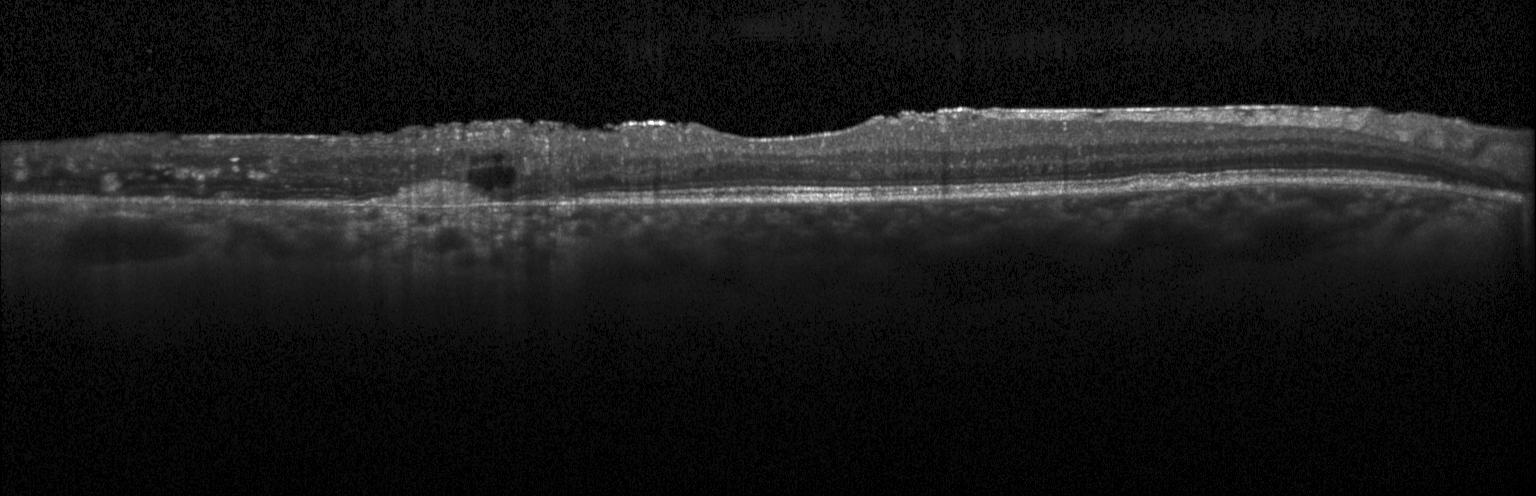
Assessment: DME.